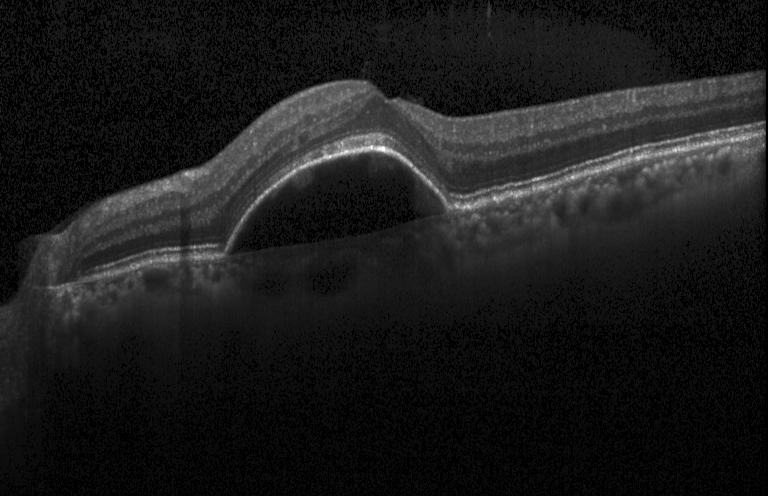
Centered on the fovea. OCT line scan — Impression: CNV.